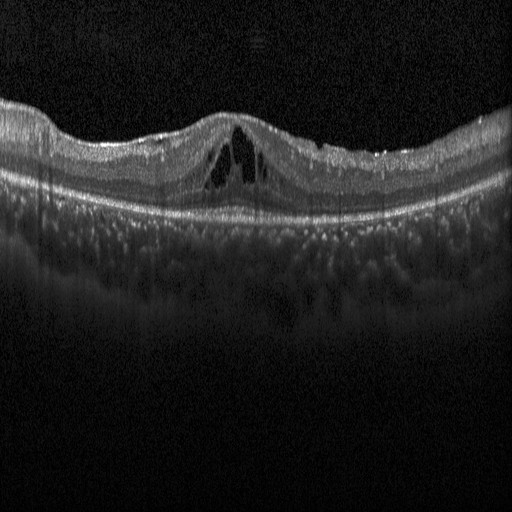
Optical coherence tomography B-scan, fovea-centered, SD-OCT, instrument: Heidelberg Spectralis
Finding: diabetic macular edema (DME).